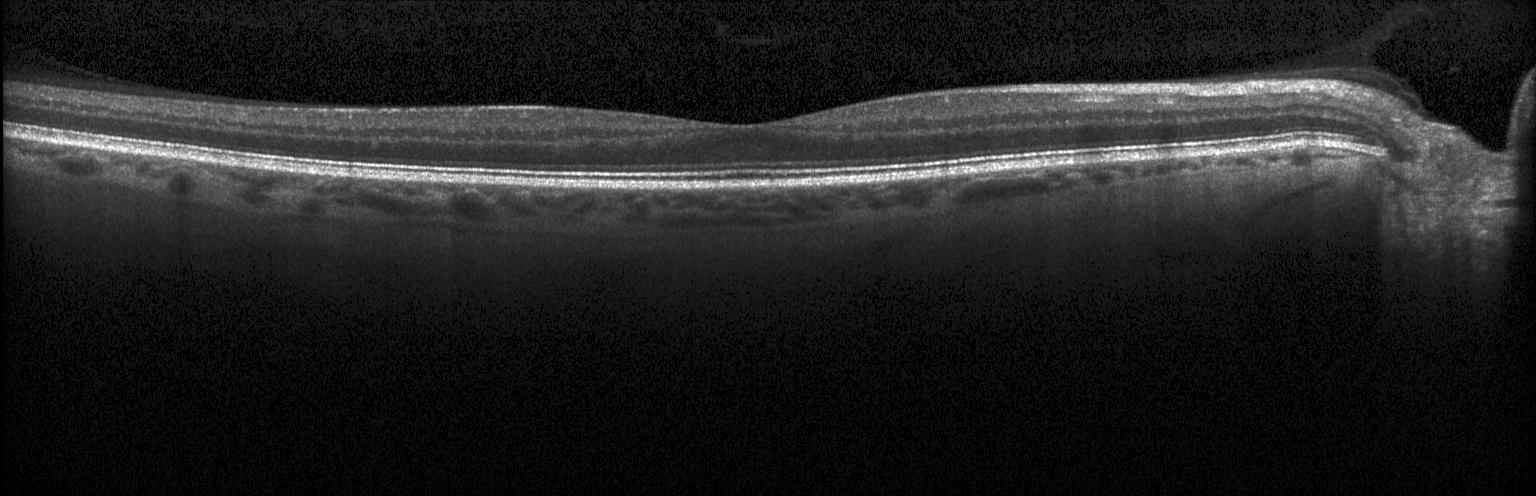

OCT scan showing no choroidal neovascularization, no diabetic macular edema, and no drusen.